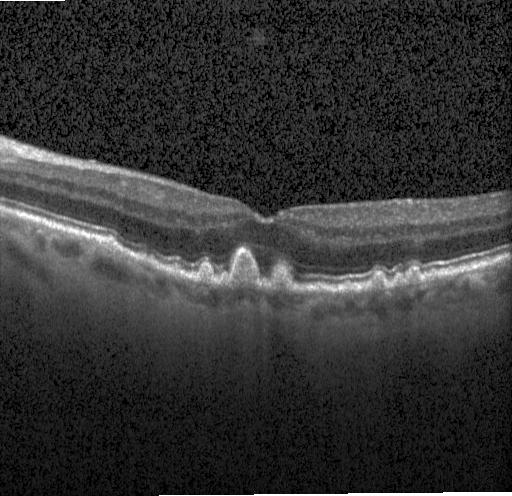
Finding: drusen.